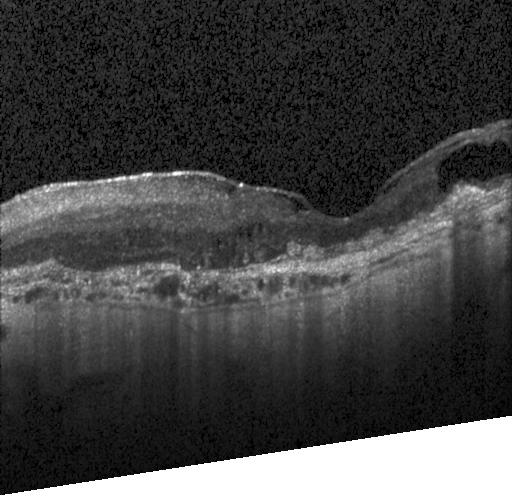 OCT line scan. Spectral-domain optical coherence tomography — Diagnosis: a choroidal neovascular membrane.